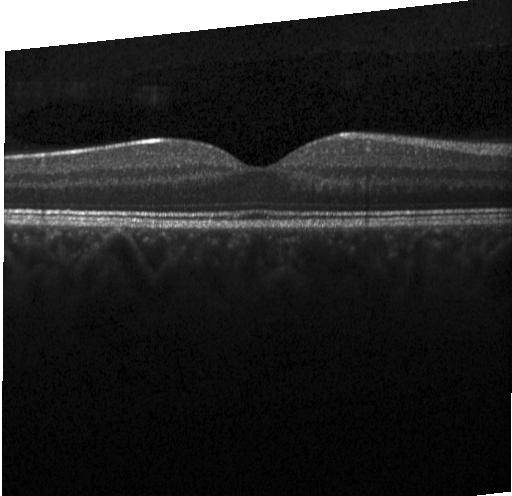 OCT B-scan.
Finding: no CNV, no DME, and no drusen.